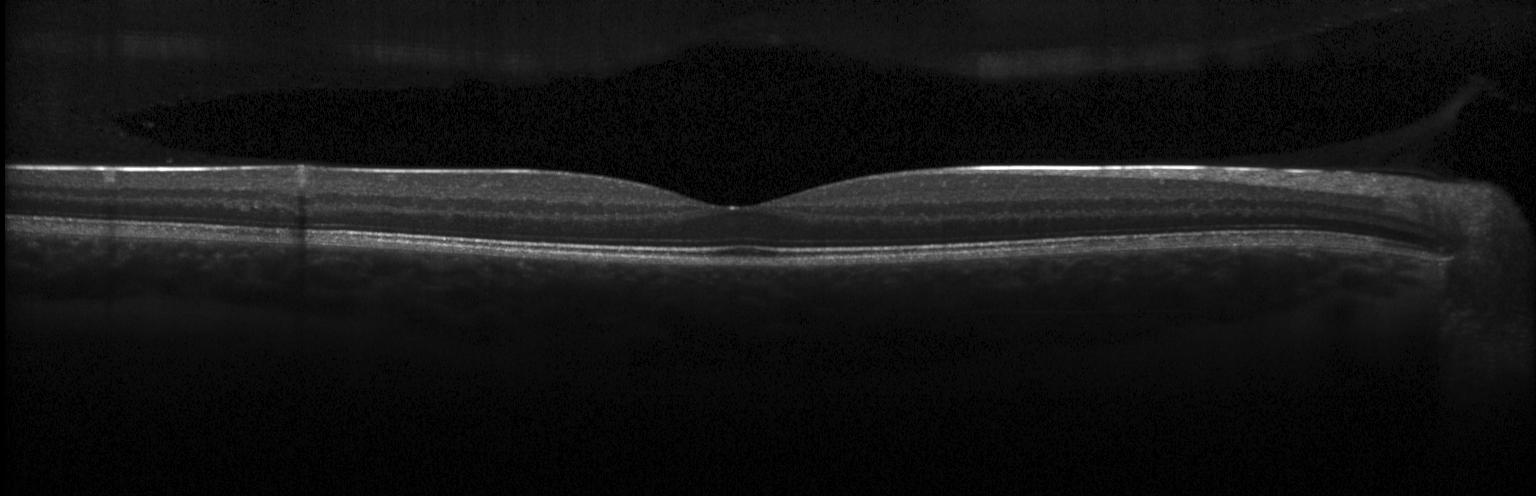

Retinal OCT cross-section. Dx: no choroidal neovascularization, diabetic macular edema, or drusen.